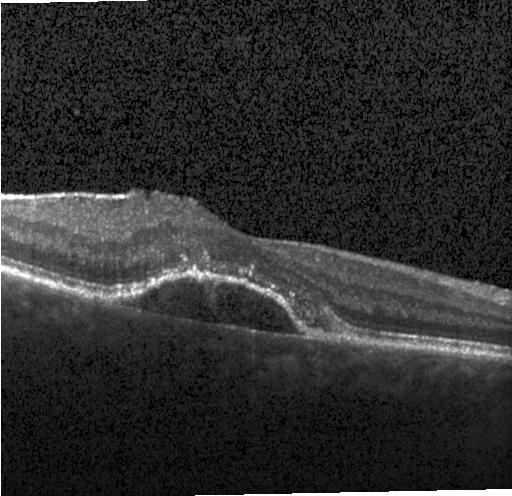
Centered on the fovea. Optical coherence tomography scan. SD-OCT.
This B-scan demonstrates a choroidal neovascular membrane.